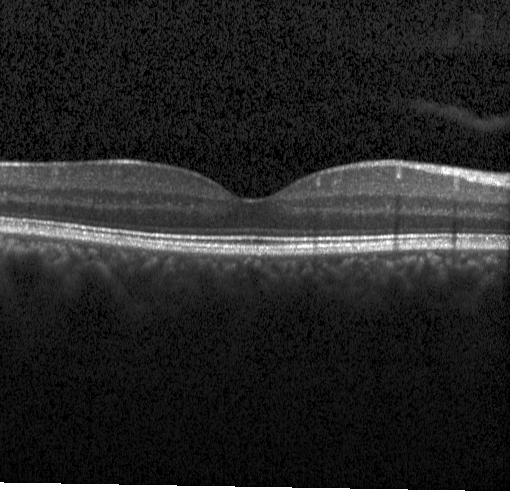 Finding: no choroidal neovascularization, no diabetic macular edema, and no drusen.